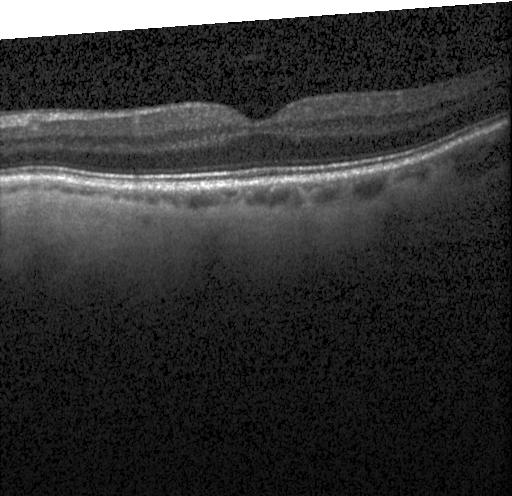 Macular OCT: no CNV, DME, or drusen.